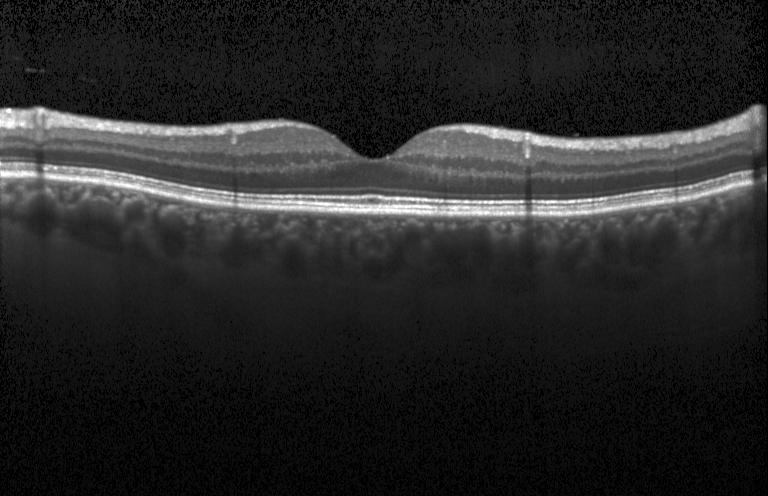

Fovea-centered · retinal OCT cross-section · acquired on a Heidelberg Spectralis. Macular OCT: no evidence of choroidal neovascularization, diabetic macular edema, or drusen.